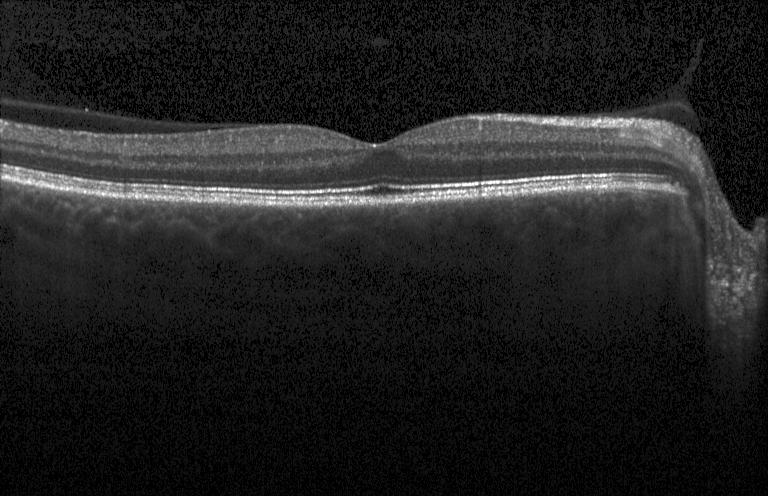

Spectral-domain OCT B-scan: no choroidal neovascularization, no diabetic macular edema, and no drusen.